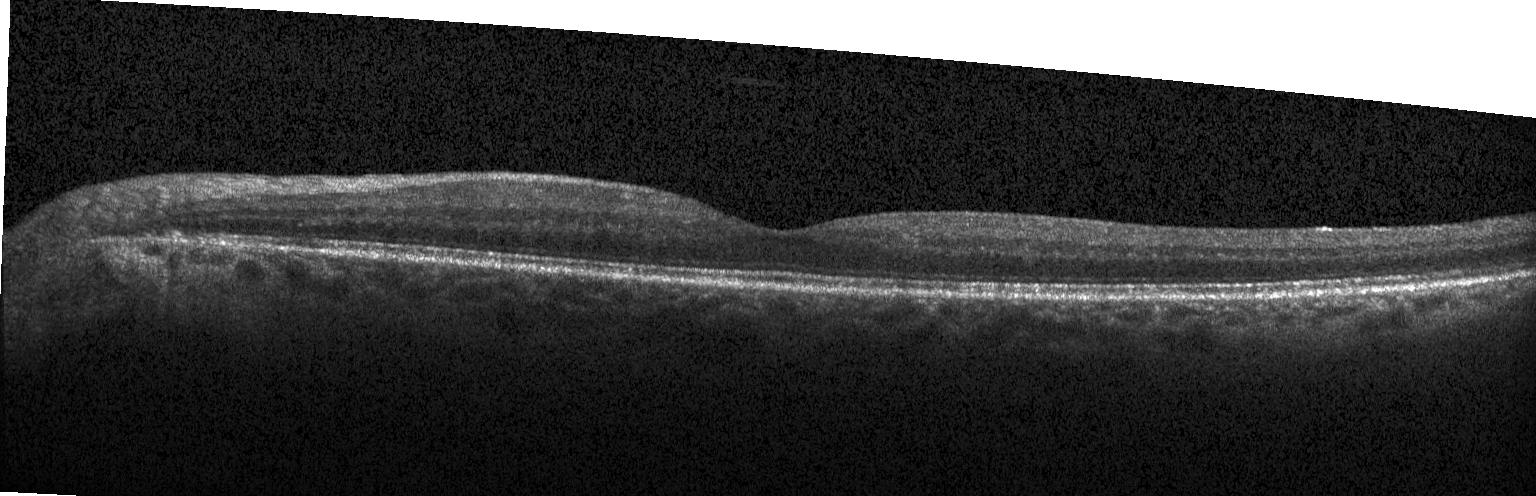
OCT scan showing no evidence of choroidal neovascularization, diabetic macular edema, or drusen.